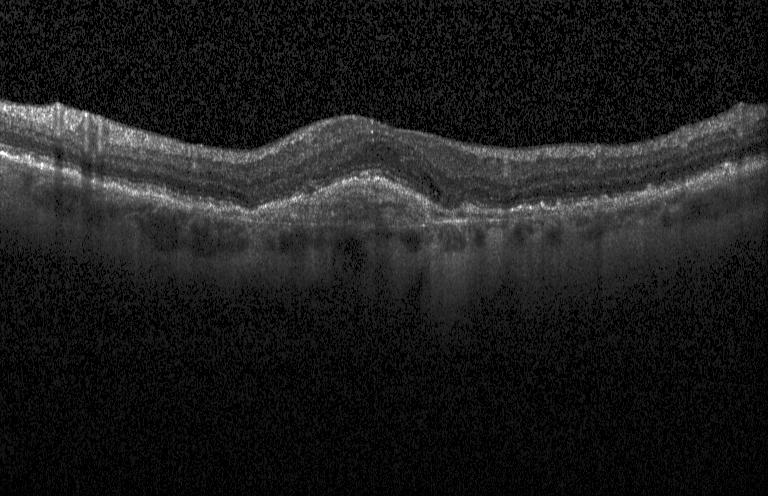
SD-OCT; retinal OCT cross-section.
Impression: a choroidal neovascular membrane.